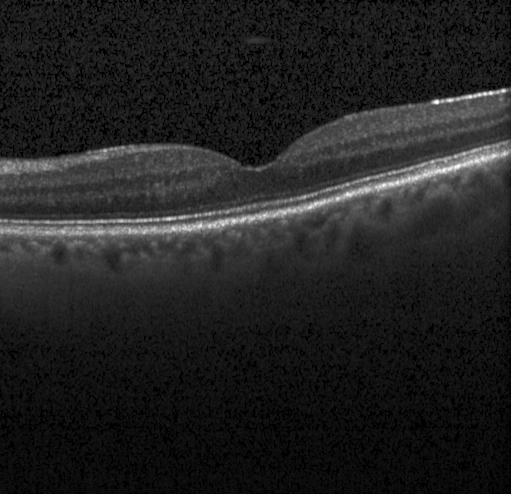
Dx: neither CNV, DME, nor drusen.